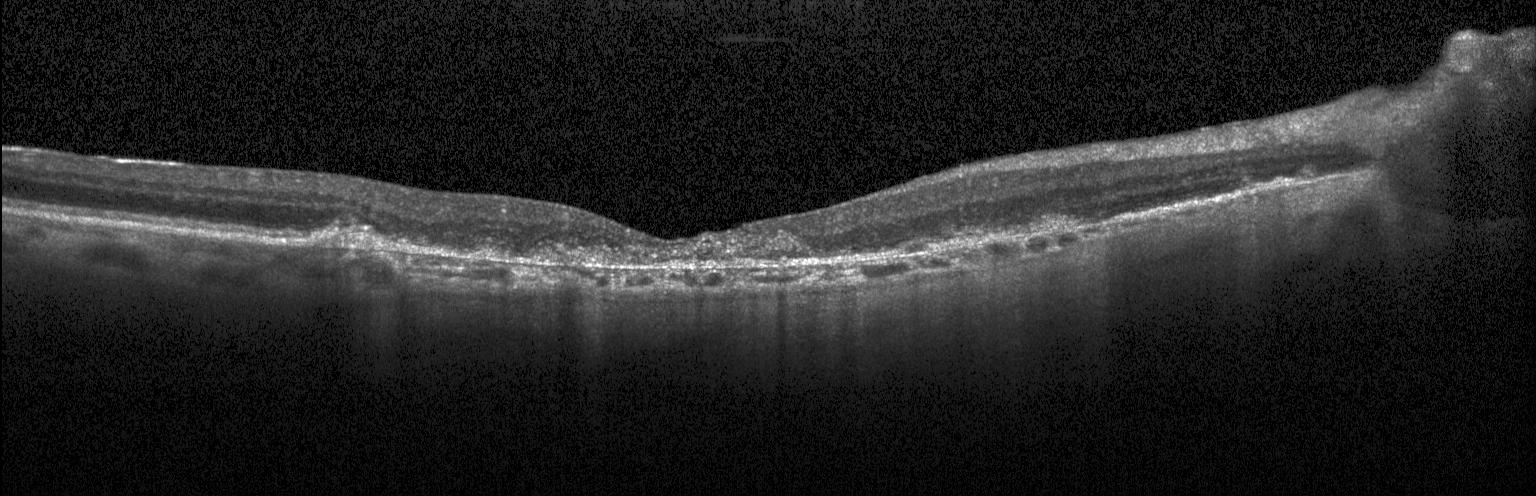

Centered on the fovea · retinal OCT cross-section — Assessment: a choroidal neovascular membrane.